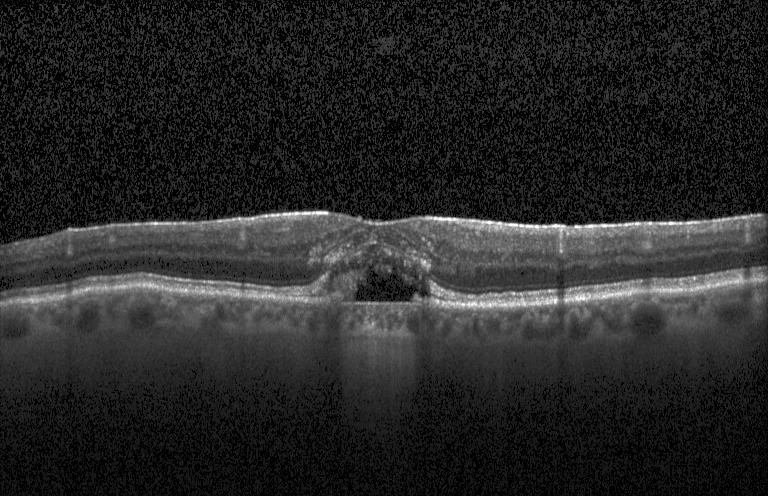
Assessment: a choroidal neovascular membrane.